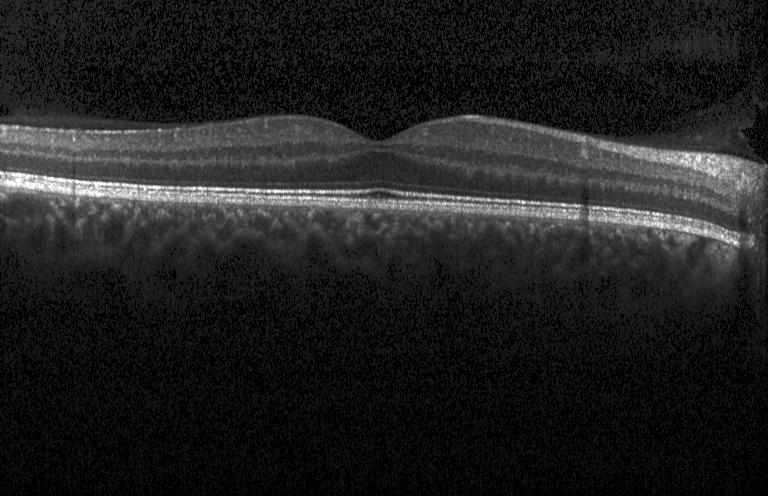 Fovea-centered · SD-OCT · OCT B-scan · instrument: Heidelberg Spectralis. No choroidal neovascularization, no diabetic macular edema, and no drusen.